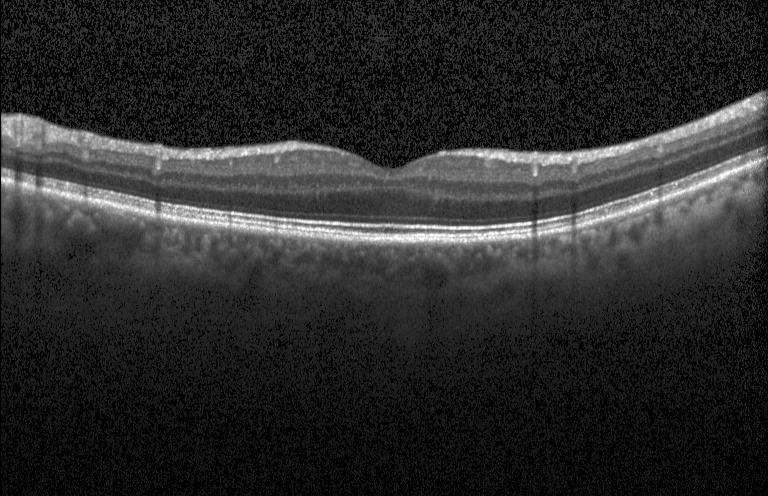

Optical coherence tomography scan. This B-scan demonstrates no CNV, DME, or drusen.